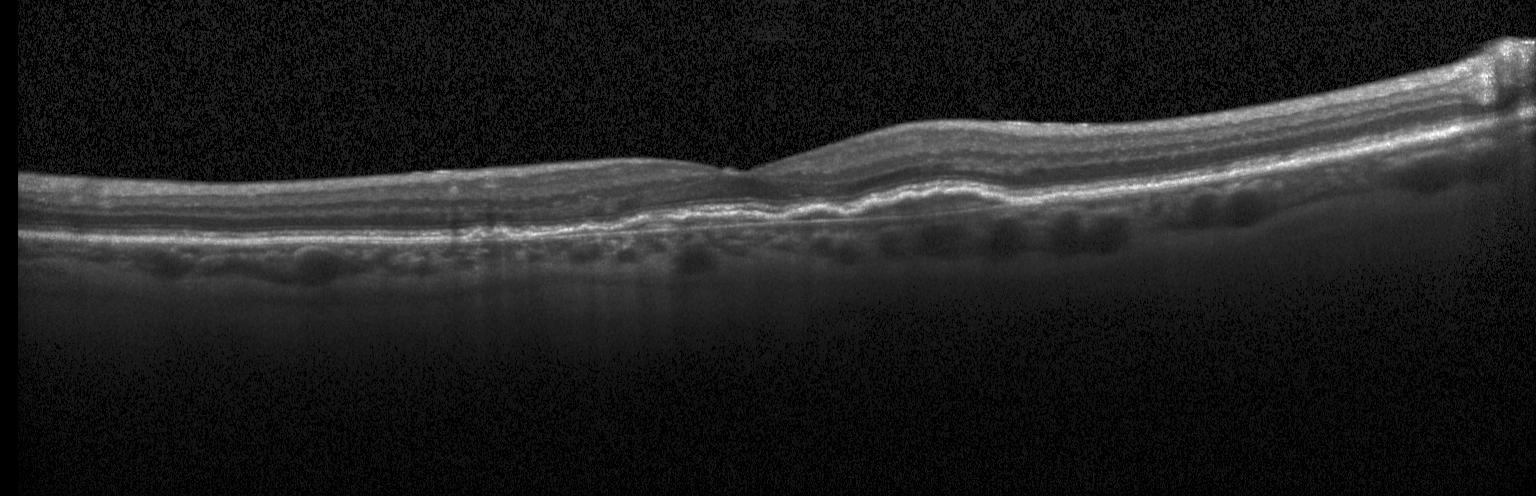

Spectral-domain optical coherence tomography. Optical coherence tomography B-scan. Macular scan. Diagnosis: choroidal neovascularization.